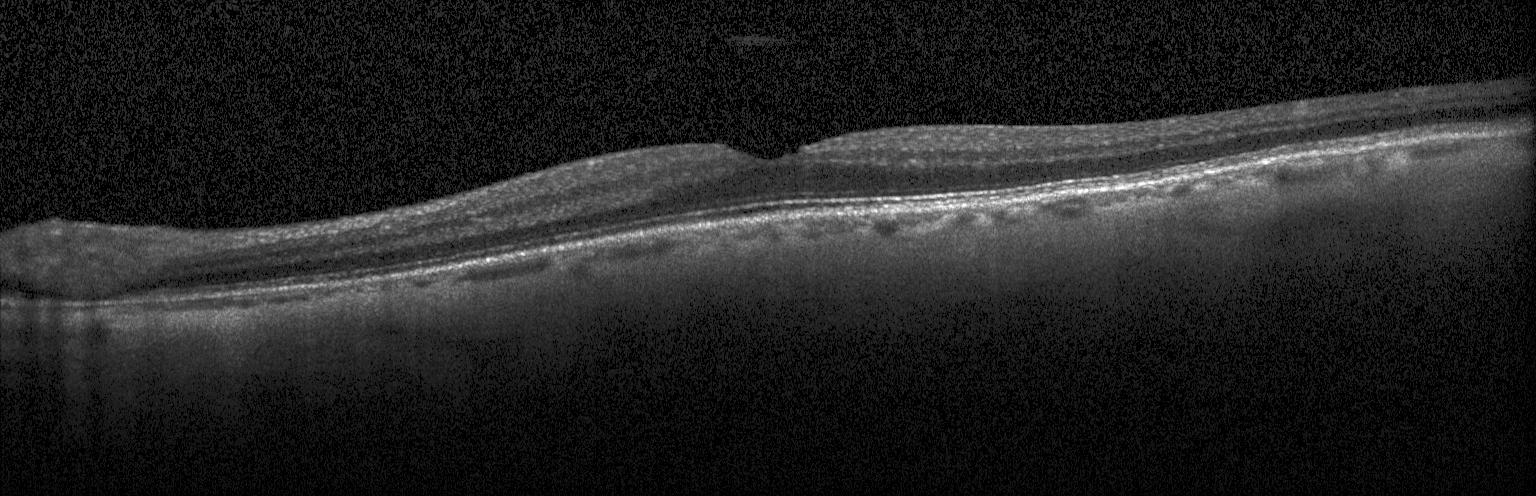
Instrument: Heidelberg Spectralis · optical coherence tomography B-scan
Assessment: no choroidal neovascularization, no diabetic macular edema, and no drusen.